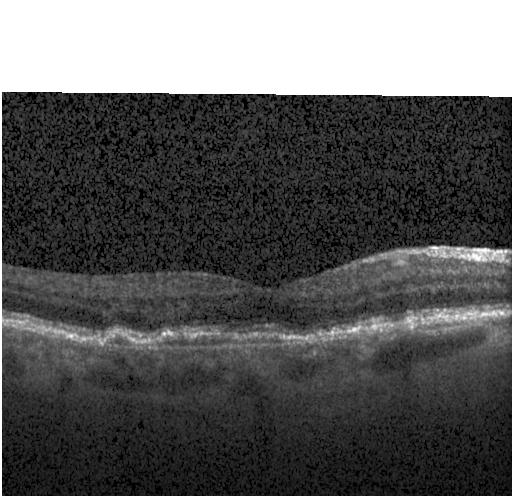 Spectral-domain OCT B-scan: a choroidal neovascular membrane.